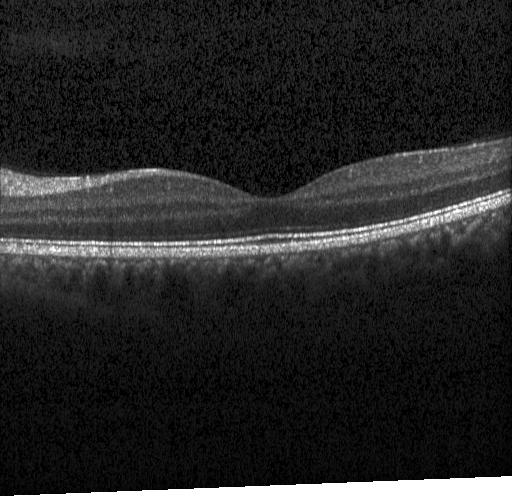 The scan shows no choroidal neovascularization, diabetic macular edema, or drusen.